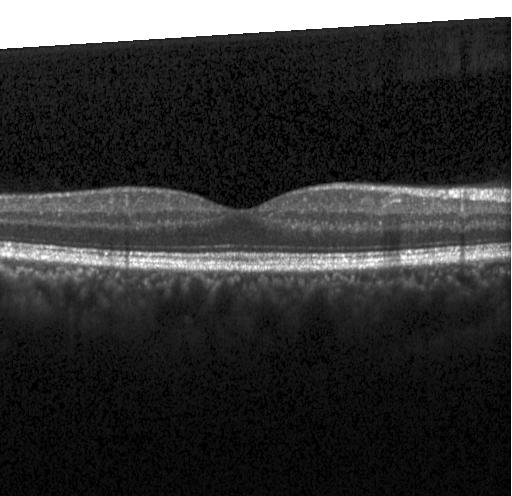

Retinal OCT cross-section, Heidelberg Spectralis OCT system. This B-scan demonstrates no choroidal neovascularization, diabetic macular edema, or drusen.